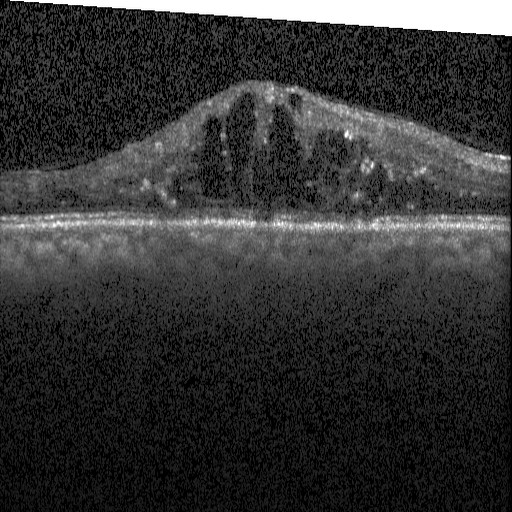

Optical coherence tomography B-scan
Finding: DME.